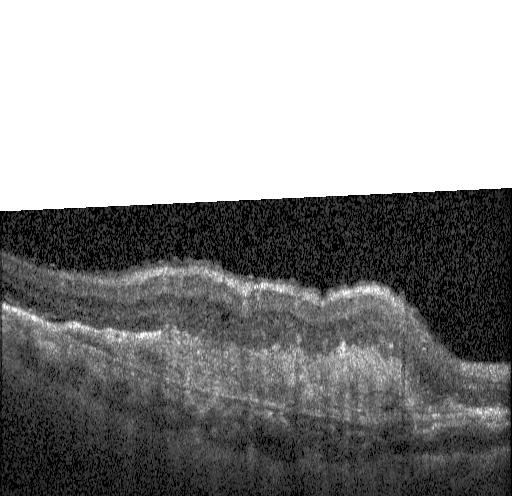
Optical coherence tomography B-scan; macular scan; SD-OCT.
Finding: a choroidal neovascular membrane.